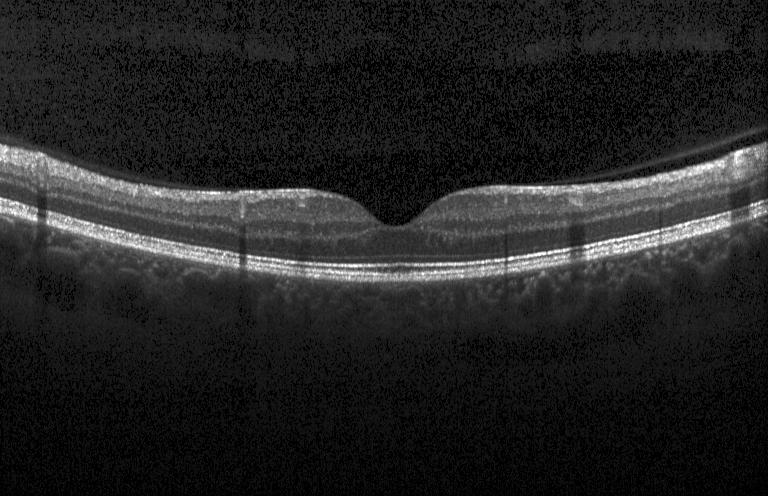 Macular OCT demonstrating no CNV, DME, or drusen.